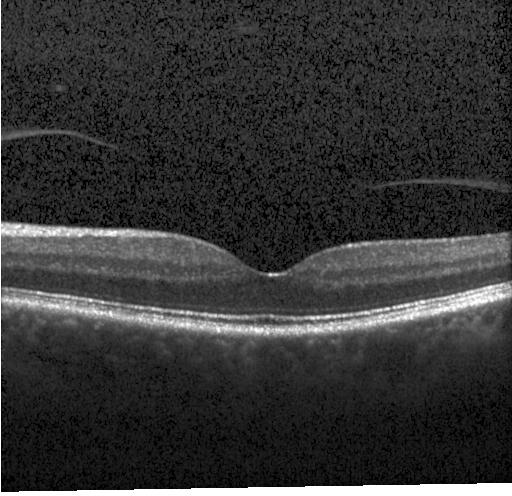 OCT scan showing no choroidal neovascularization, diabetic macular edema, or drusen.